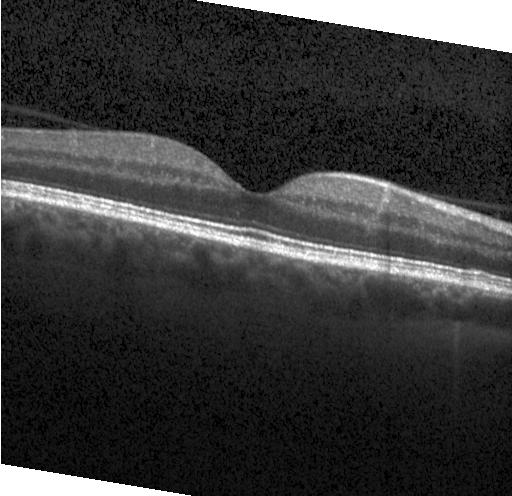
Spectral-domain optical coherence tomography; retinal OCT cross-section — OCT finding: neither choroidal neovascularization, diabetic macular edema, nor drusen.